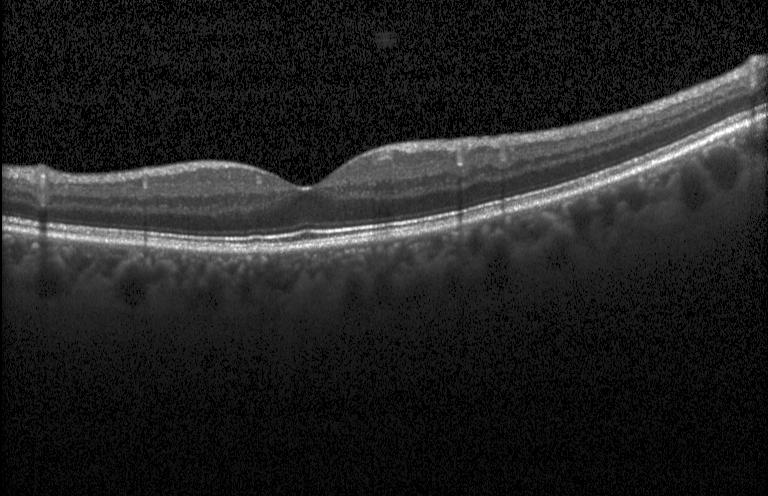 Optical coherence tomography scan · SD-OCT. Finding: no CNV, no DME, and no drusen.